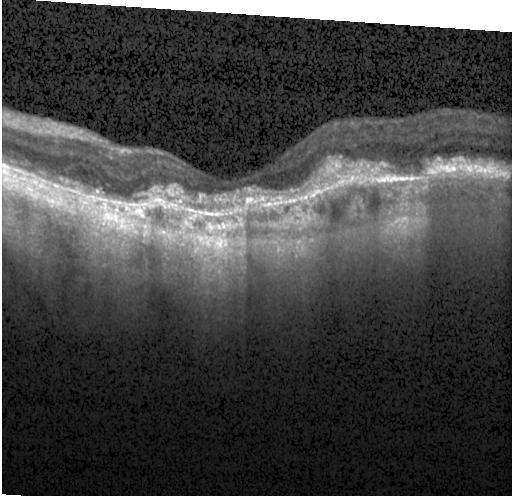

Retinal OCT B-scan — Diagnosis: choroidal neovascularization (CNV).